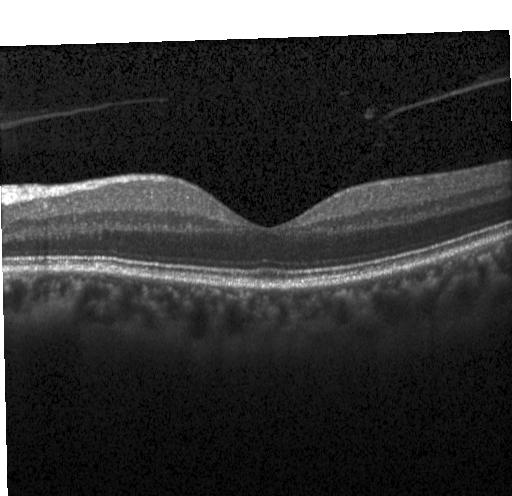

Instrument: Heidelberg Spectralis, OCT line scan, horizontal scan through the fovea. Impression: no choroidal neovascularization, diabetic macular edema, or drusen.